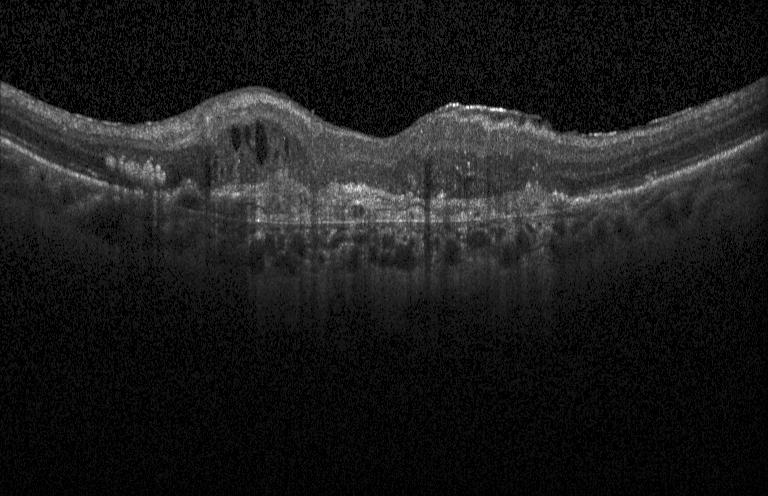
OCT finding: CNV.